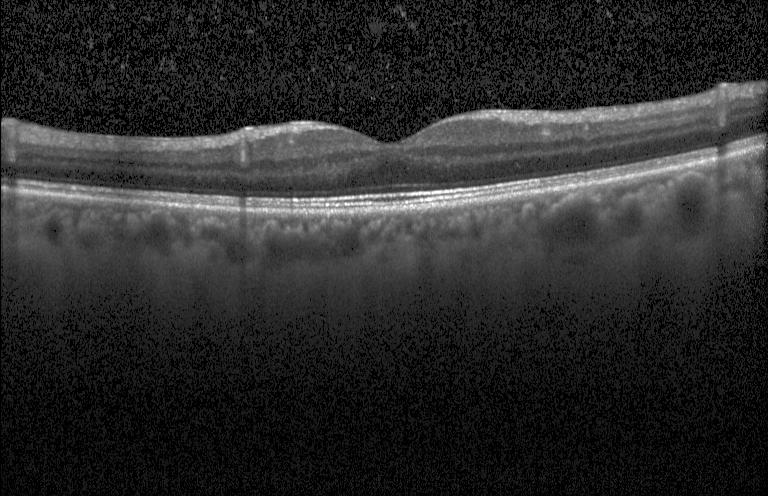
OCT B-scan showing no choroidal neovascularization, no diabetic macular edema, and no drusen.